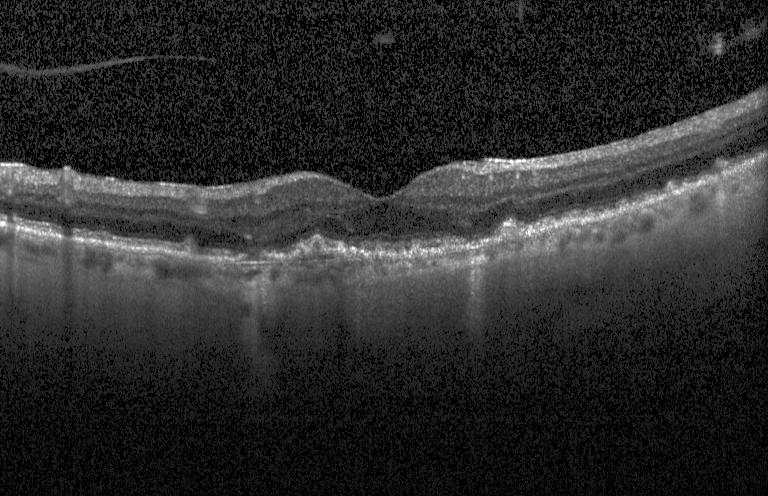

Fovea-centered. Retinal OCT B-scan. Heidelberg Spectralis.
Finding: multiple drusen.